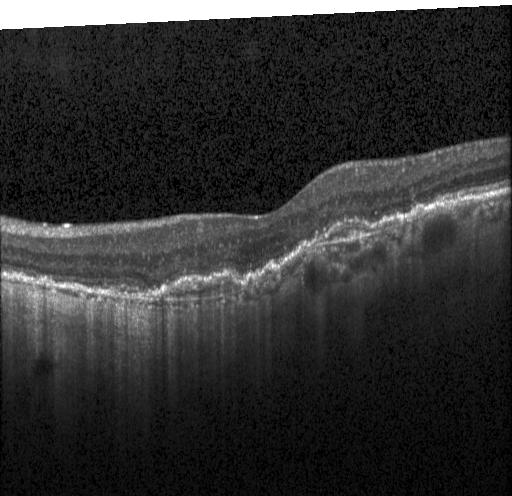 Retinal OCT B-scan; spectral-domain optical coherence tomography. Impression: a choroidal neovascular membrane.